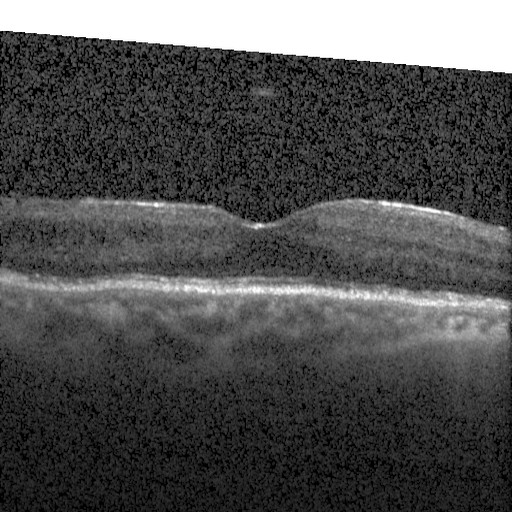
OCT B-scan · fovea-centered · spectral-domain optical coherence tomography.
Impression: diabetic macular edema (DME).